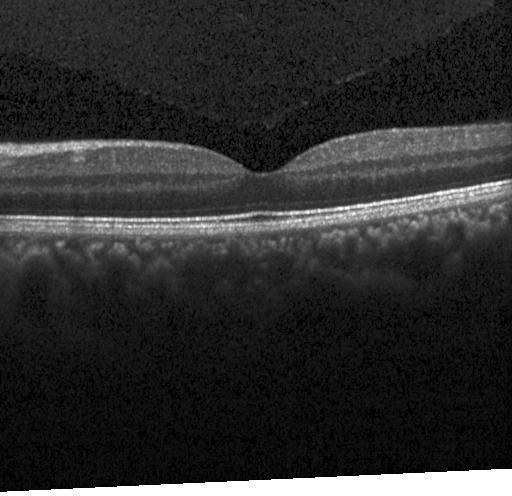
OCT line scan
No evidence of CNV, DME, or drusen.